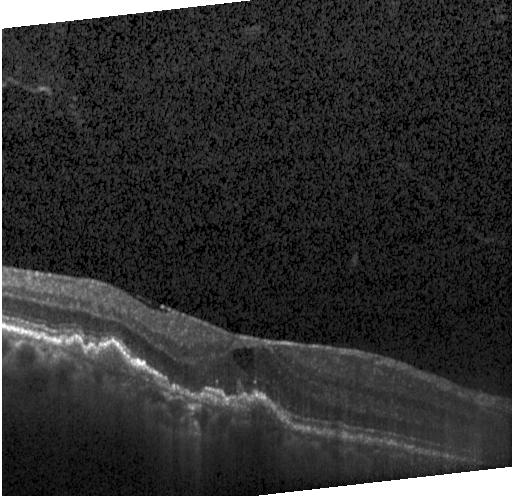 Retinal OCT B-scan, macular scan, instrument: Heidelberg Spectralis. Macular OCT: CNV.